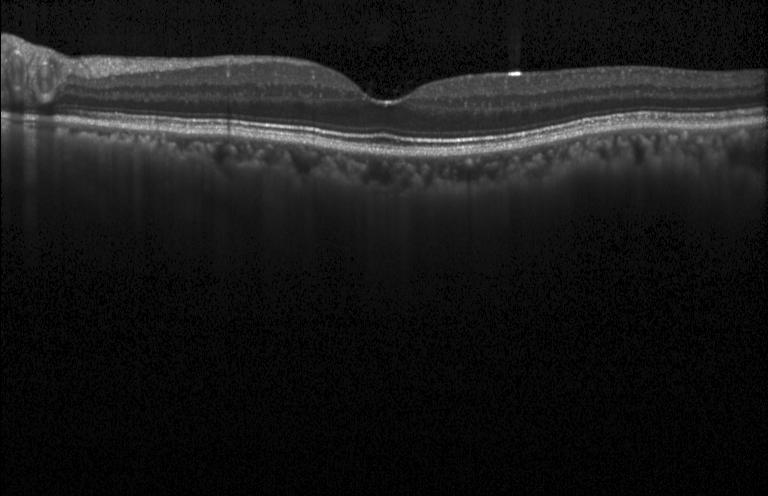

Spectral-domain OCT, optical coherence tomography B-scan, through the macula
Diagnosis: no CNV, DME, or drusen.